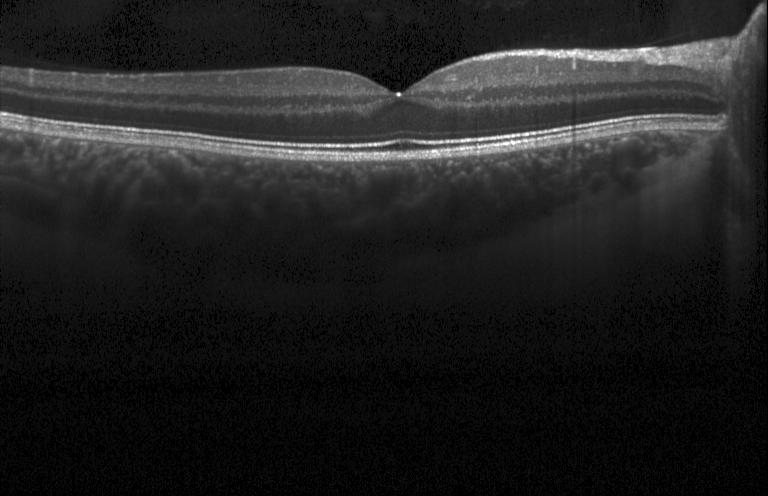
Optical coherence tomography scan. Dx: neither CNV, DME, nor drusen.